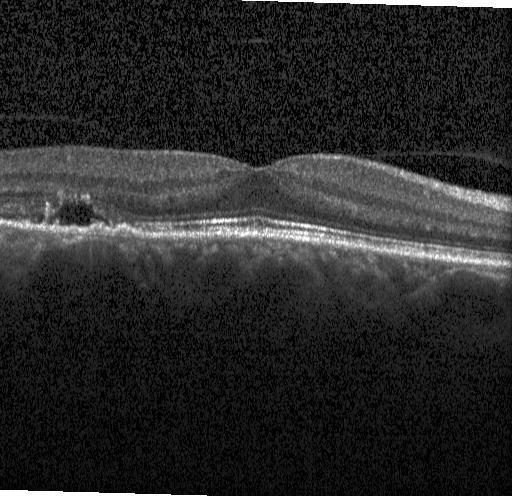
Spectral-domain OCT, acquired on a Heidelberg Spectralis, centered on the fovea, optical coherence tomography scan — Finding: a choroidal neovascular membrane.